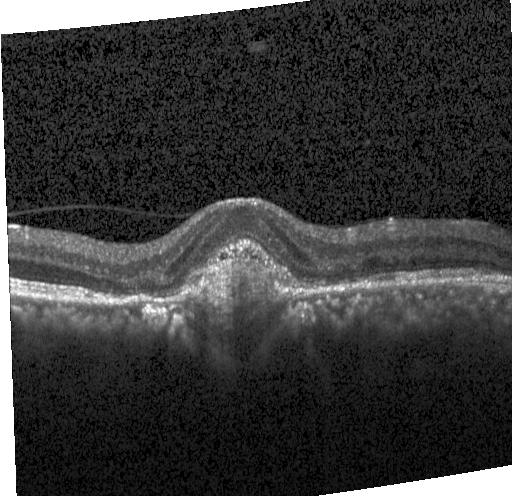 Diagnosis: a choroidal neovascular membrane.